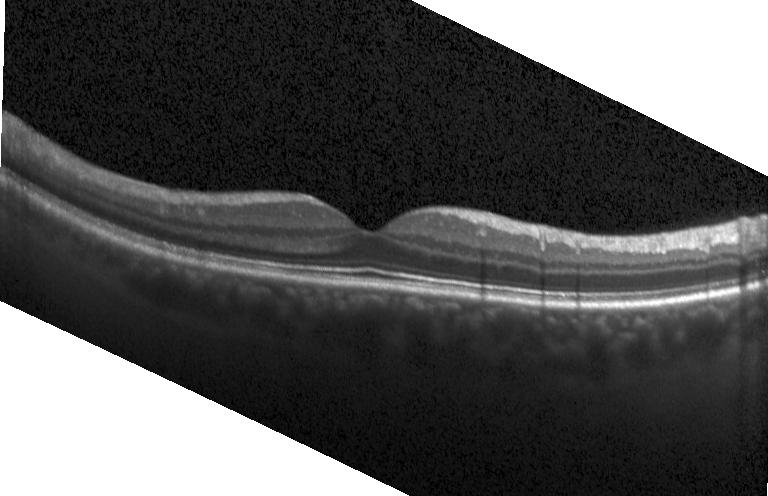

Centered on the fovea. Optical coherence tomography B-scan. The scan shows no CNV, DME, or drusen.